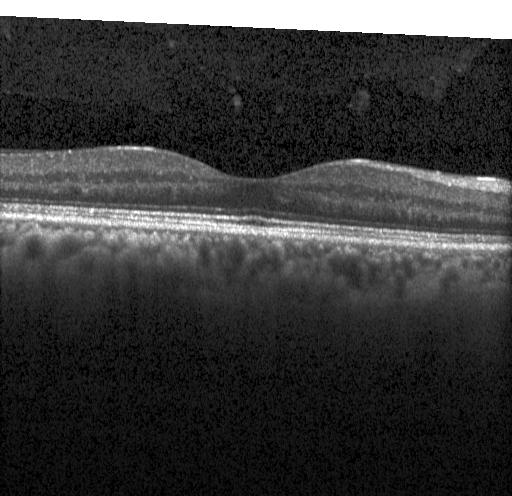
OCT B-scan — Diagnosis: no choroidal neovascularization, diabetic macular edema, or drusen.